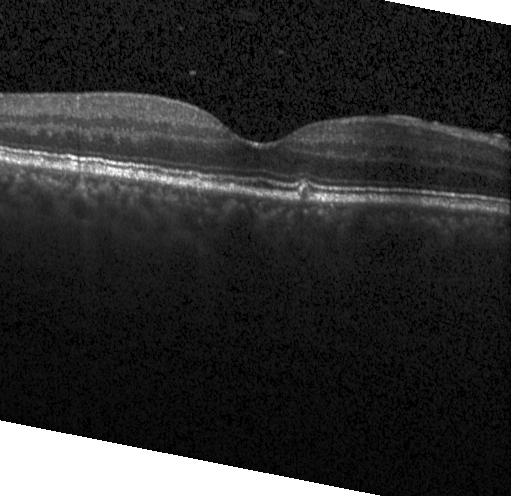 Heidelberg Spectralis, retinal OCT cross-section, spectral-domain optical coherence tomography.
Dx: multiple drusen.